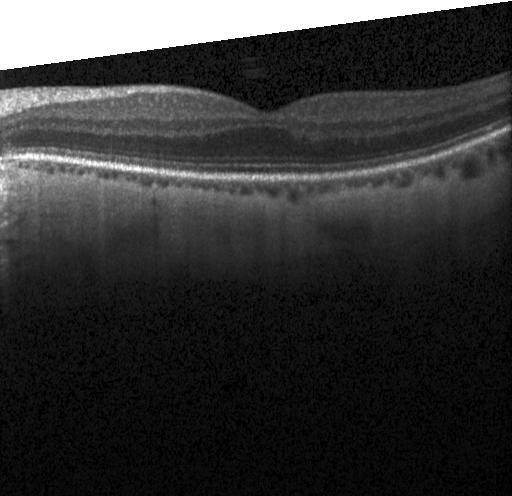
Optical coherence tomography B-scan. Centered on the fovea. Spectral-domain OCT. Heidelberg Spectralis
Dx: no choroidal neovascularization, no diabetic macular edema, and no drusen.